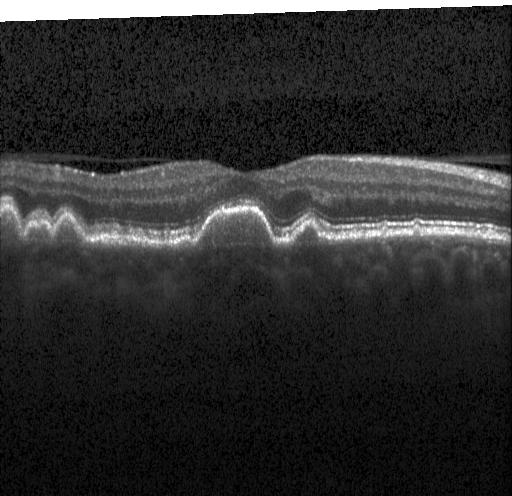

Optical coherence tomography B-scan; SD-OCT
Finding: multiple drusen.